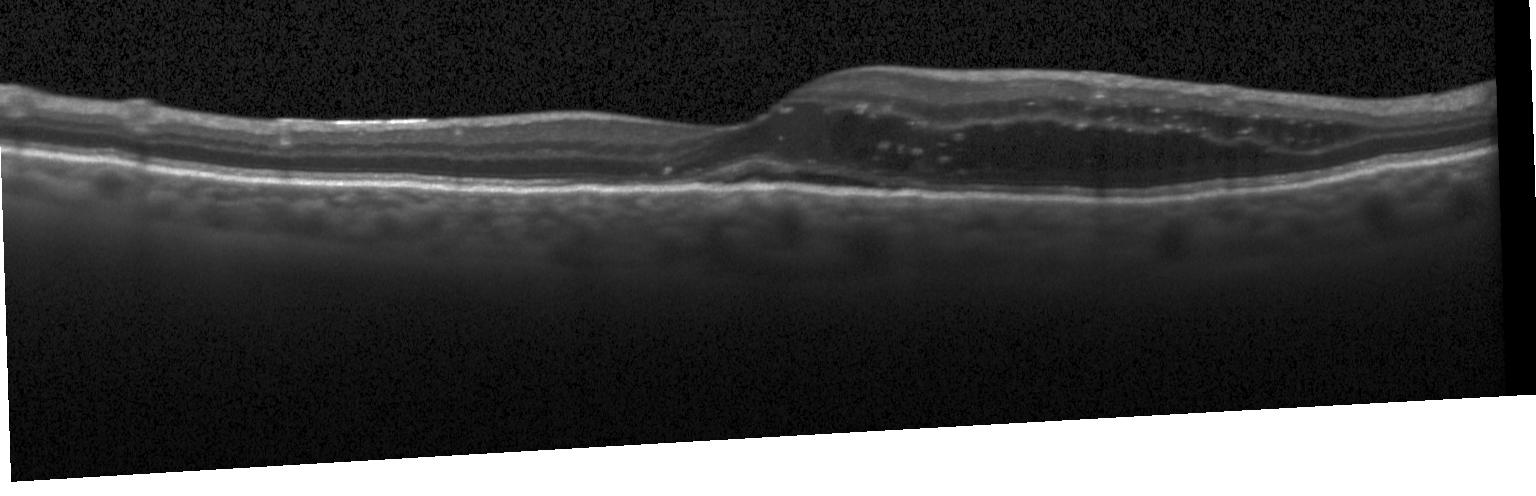
OCT line scan. Acquired on a Heidelberg Spectralis
The scan shows diabetic macular edema (DME).